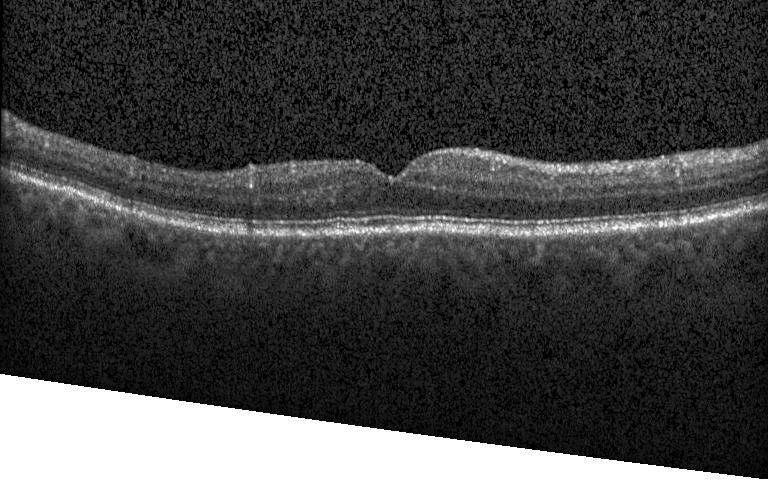

Optical coherence tomography scan · spectral-domain OCT · acquired on a Heidelberg Spectralis.
Macular OCT: no evidence of CNV, DME, or drusen.